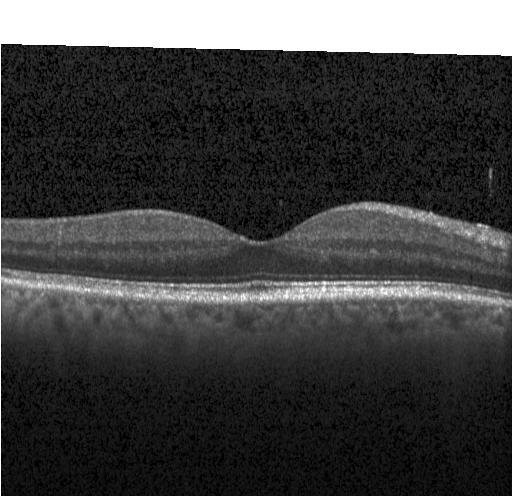 Optical coherence tomography B-scan. Fovea-centered. Spectral-domain optical coherence tomography. Heidelberg Spectralis OCT system — Diagnosis: no choroidal neovascularization, diabetic macular edema, or drusen.